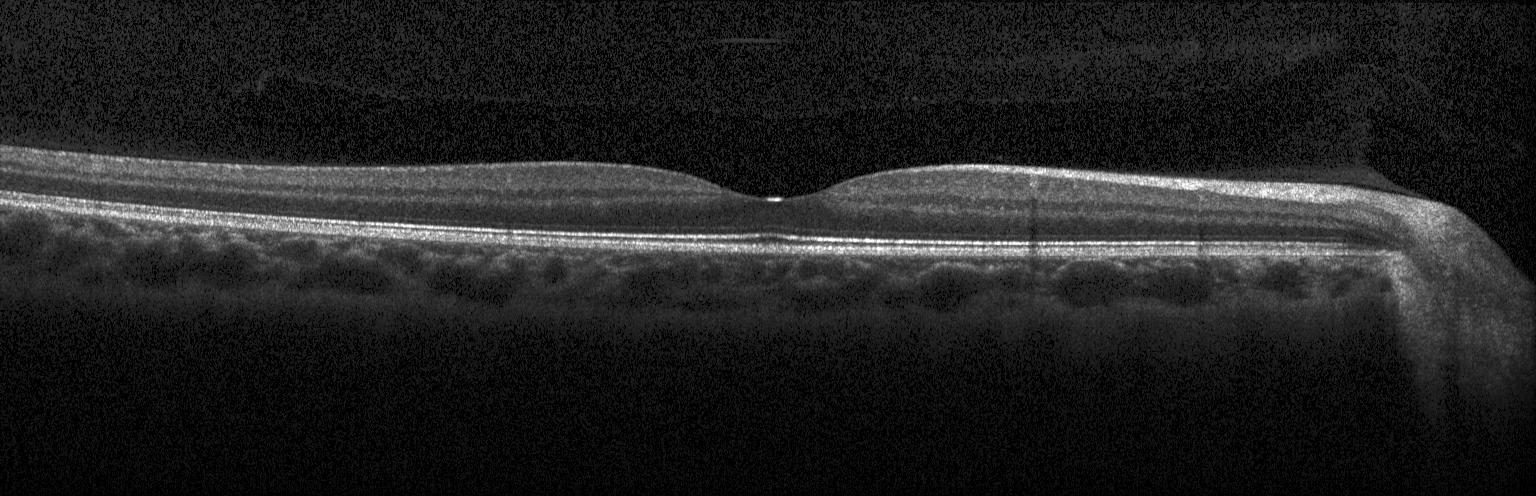 Optical coherence tomography scan; instrument: Heidelberg Spectralis; spectral-domain optical coherence tomography
Assessment: no CNV, no DME, and no drusen.